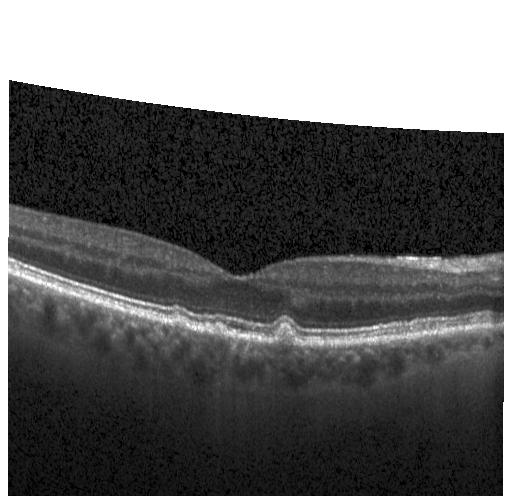 The scan shows multiple drusen.